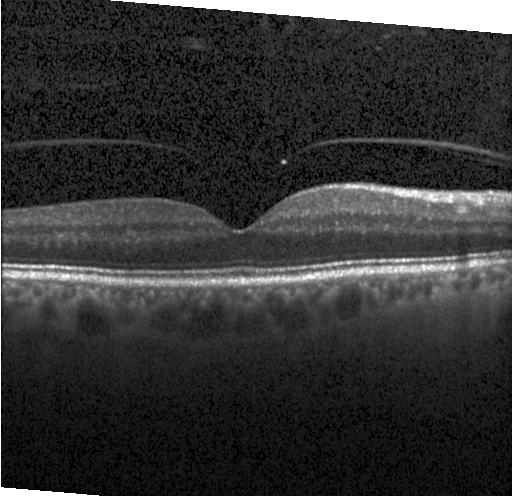
Optical coherence tomography scan
The scan shows no CNV, no DME, and no drusen.